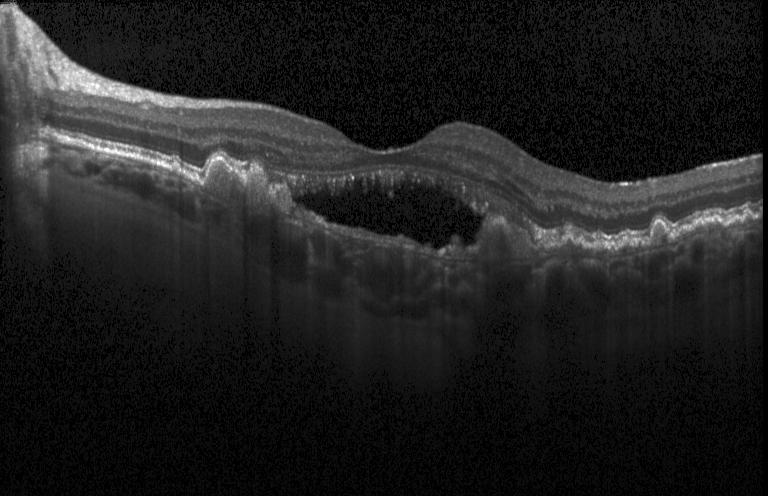
SD-OCT, retinal OCT B-scan.
The scan shows a choroidal neovascular membrane.